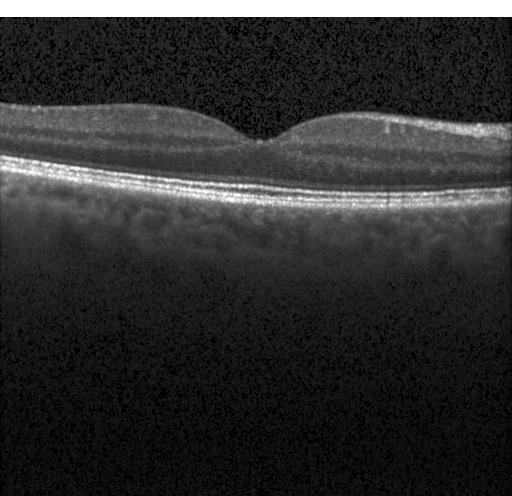
OCT line scan, spectral-domain OCT, Heidelberg Spectralis OCT system, horizontal scan through the fovea
Impression: no choroidal neovascularization, no diabetic macular edema, and no drusen.